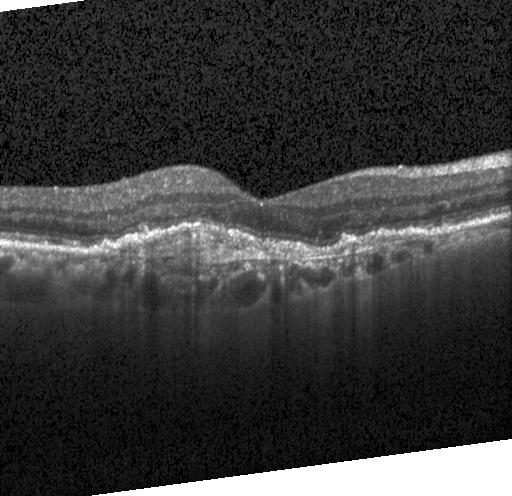

Retinal OCT B-scan — Impression: a choroidal neovascular membrane.